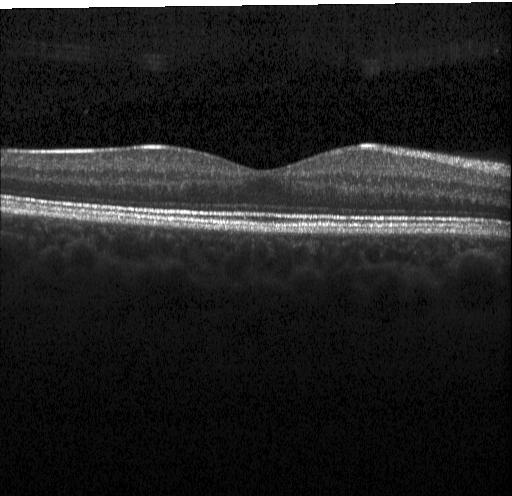 Retinal OCT cross-section · horizontal scan through the fovea · instrument: Heidelberg Spectralis · SD-OCT — Impression: no evidence of choroidal neovascularization, diabetic macular edema, or drusen.